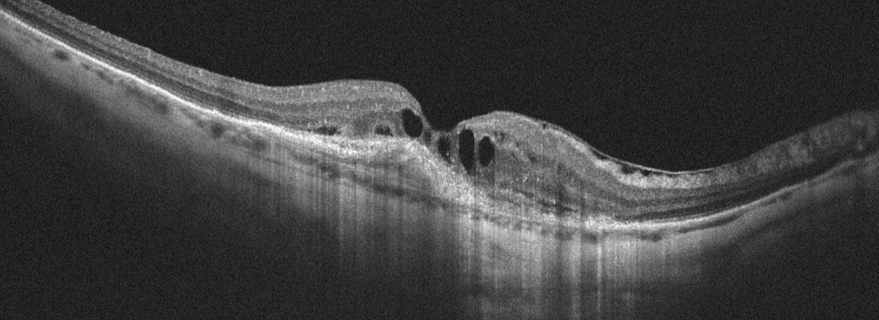

OCT line scan. Finding: age-related macular degeneration.